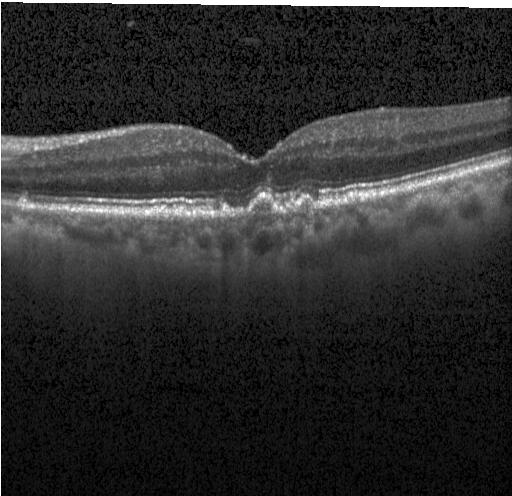
Macular OCT: drusen.